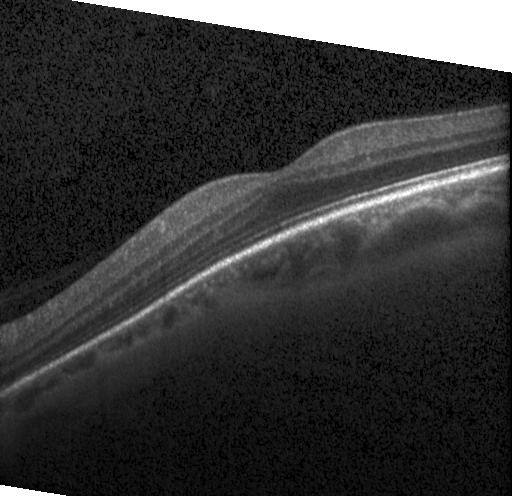

Spectral-domain OCT B-scan: no evidence of CNV, DME, or drusen.